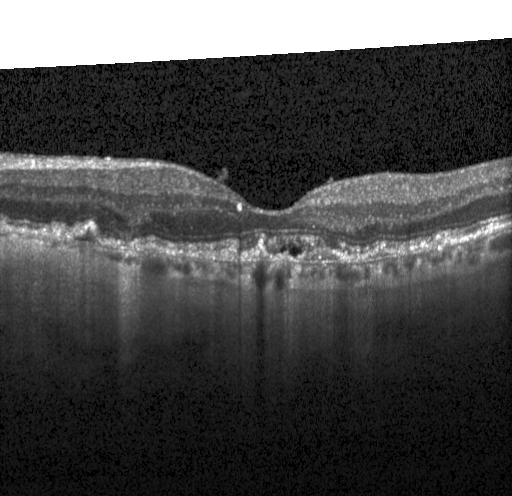
Macular scan; retinal OCT B-scan; instrument: Heidelberg Spectralis; SD-OCT
Finding: choroidal neovascularization.